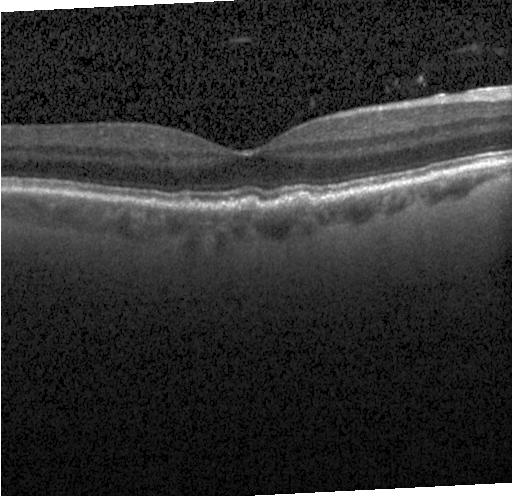
Finding: multiple drusen.